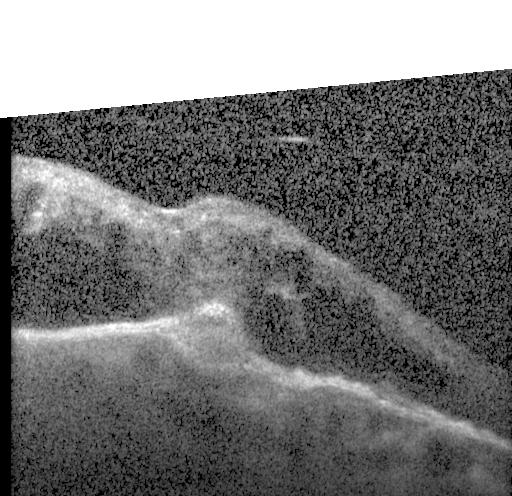 OCT B-scan — Macular OCT: a choroidal neovascular membrane.